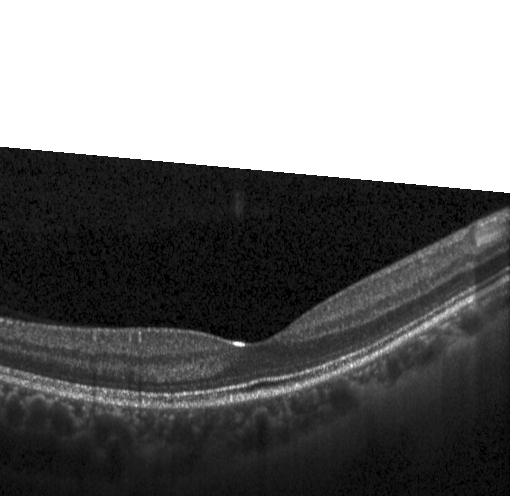

Diagnosis: no evidence of choroidal neovascularization, diabetic macular edema, or drusen.